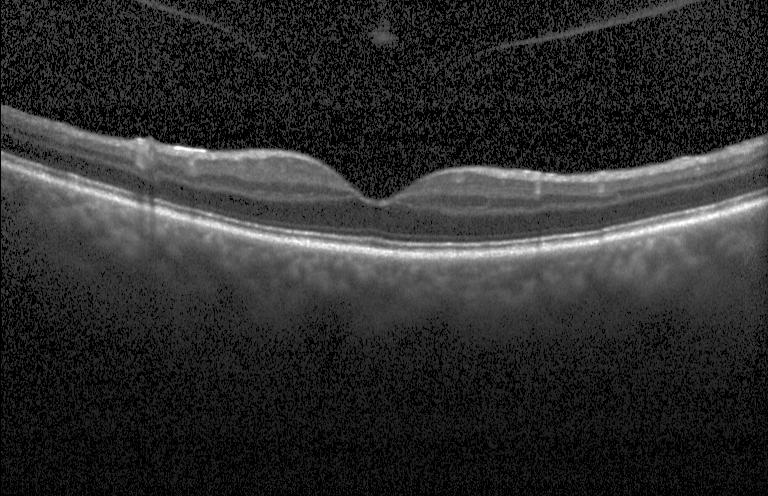

Spectral-domain OCT. Fovea-centered. Acquired on a Heidelberg Spectralis. OCT line scan — The scan shows no choroidal neovascularization, no diabetic macular edema, and no drusen.